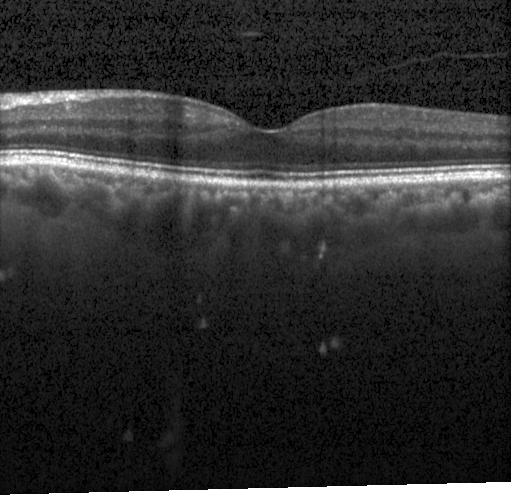
Diagnosis: neither choroidal neovascularization, diabetic macular edema, nor drusen.